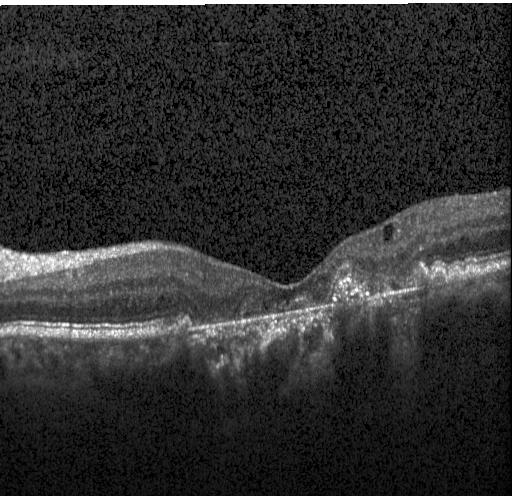 Macular OCT: choroidal neovascularization.